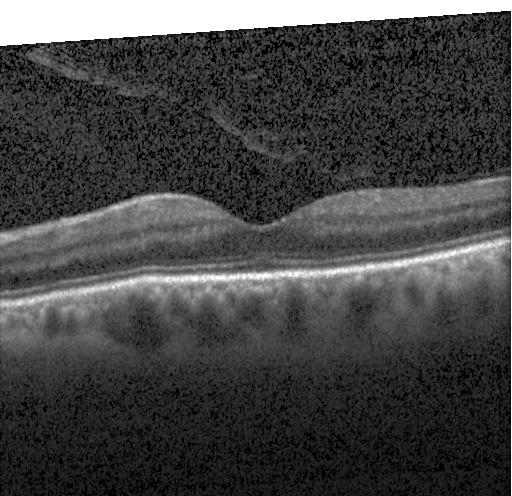
Heidelberg Spectralis · centered on the fovea · OCT line scan · spectral-domain optical coherence tomography.
Macular OCT: neither choroidal neovascularization, diabetic macular edema, nor drusen.